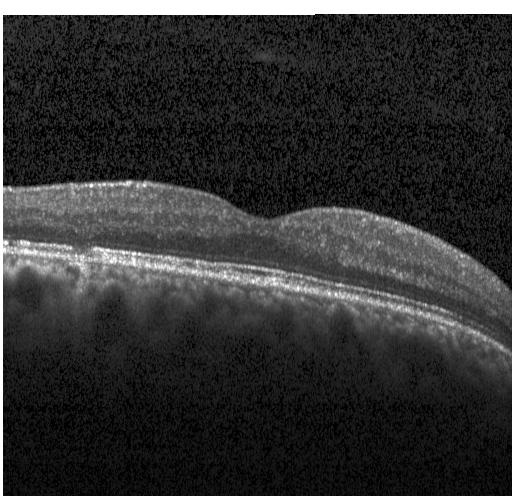

Macular OCT: no choroidal neovascularization, no diabetic macular edema, and no drusen.